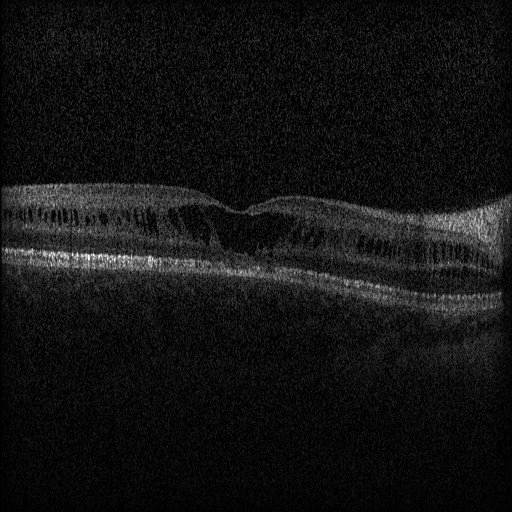

Diagnosis: diabetic macular edema.